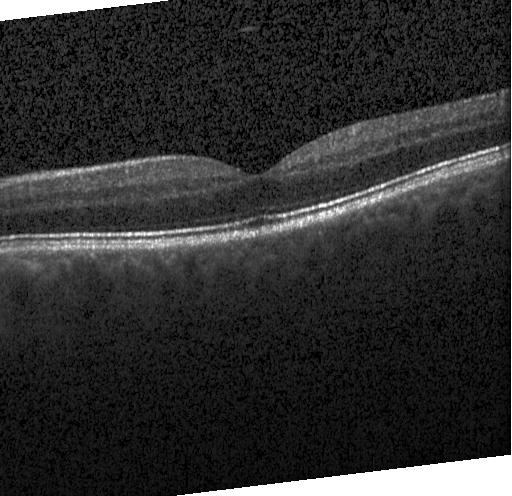
Optical coherence tomography scan. Heidelberg Spectralis OCT system. SD-OCT. Horizontal scan through the fovea. Impression: no evidence of choroidal neovascularization, diabetic macular edema, or drusen.